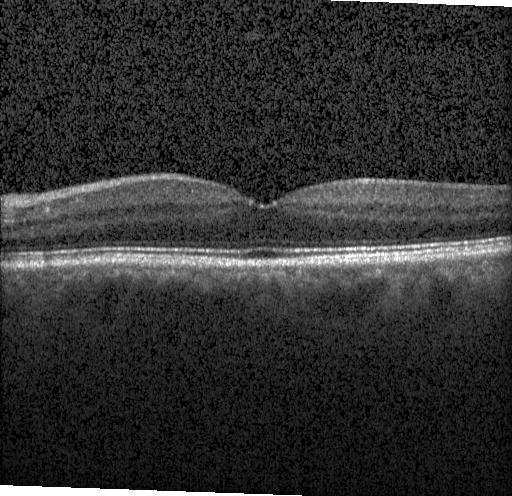
Instrument: Heidelberg Spectralis, centered on the fovea, OCT B-scan — Dx: no evidence of choroidal neovascularization, diabetic macular edema, or drusen.